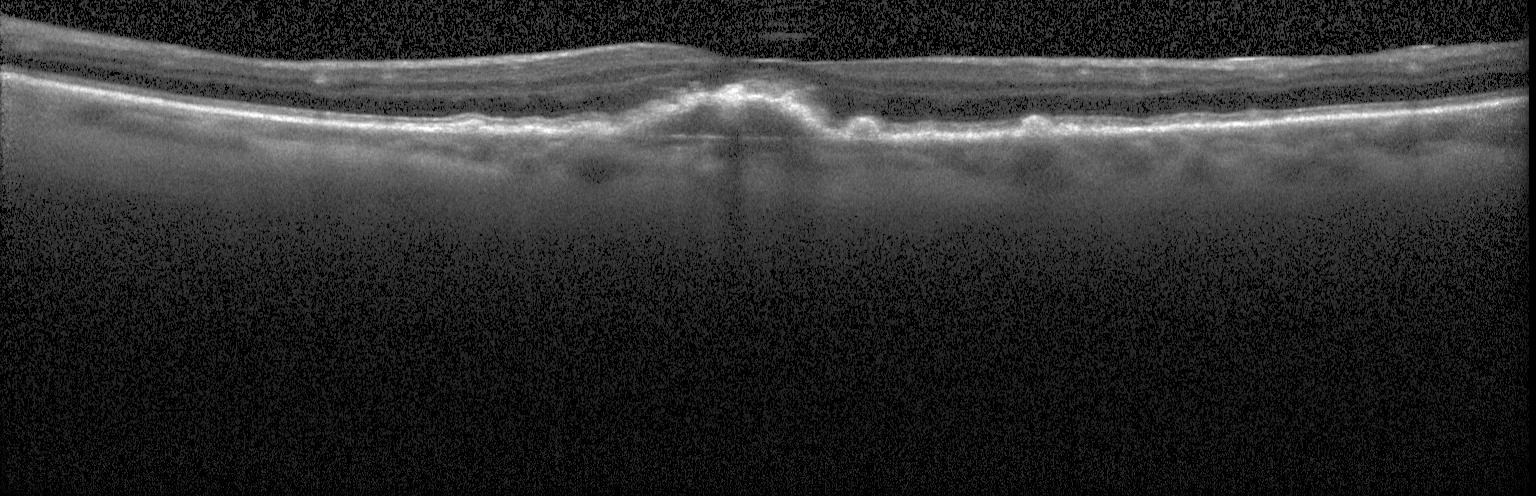

Spectral-domain OCT B-scan: choroidal neovascularization.